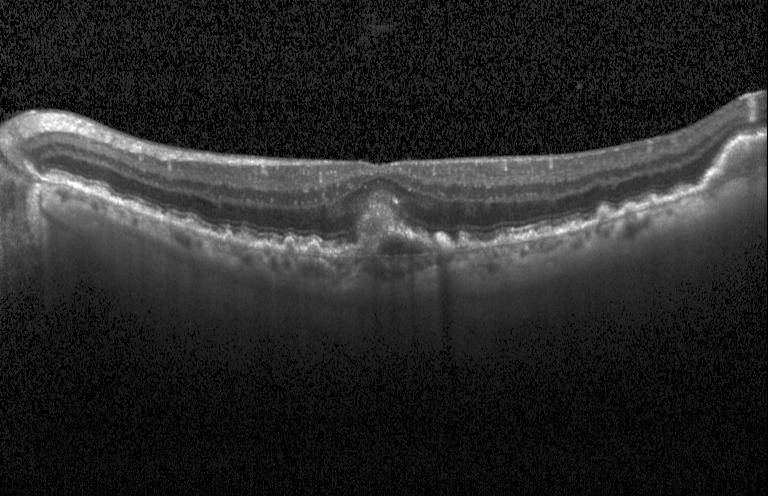 Macular OCT demonstrating CNV.